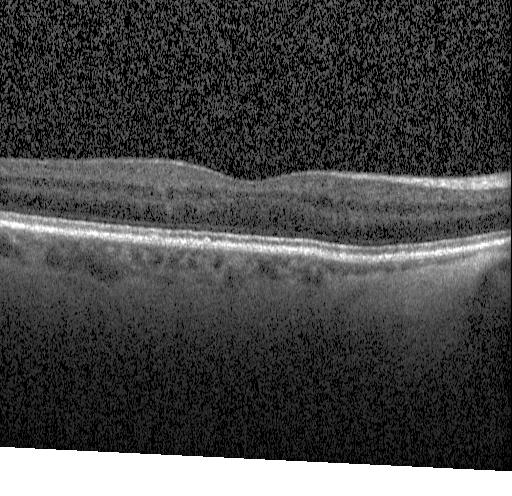 OCT B-scan — Impression: no choroidal neovascularization, no diabetic macular edema, and no drusen.